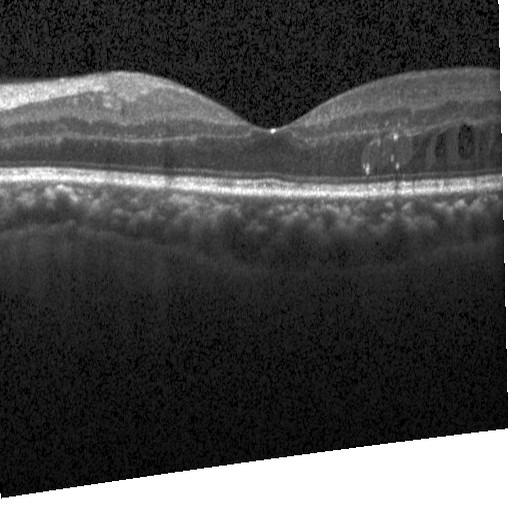 Retinal OCT cross-section; horizontal scan through the fovea
Impression: diabetic macular edema.